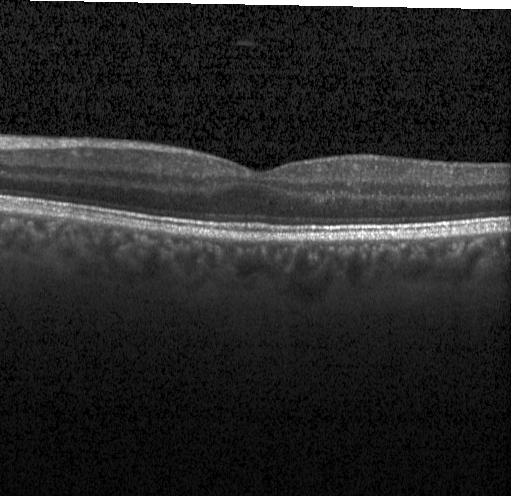

Optical coherence tomography B-scan; spectral-domain OCT — Neither choroidal neovascularization, diabetic macular edema, nor drusen.